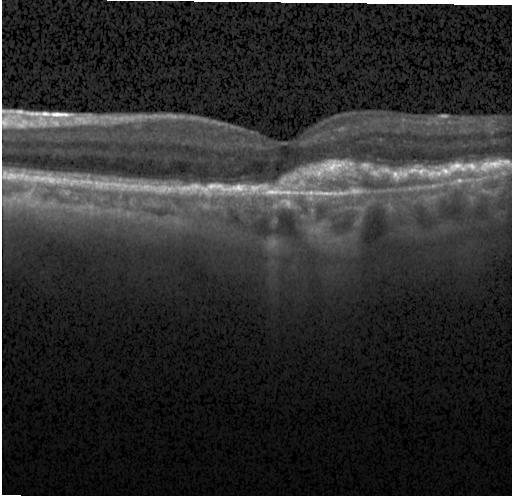
Optical coherence tomography B-scan. Macular scan
Assessment: a choroidal neovascular membrane.